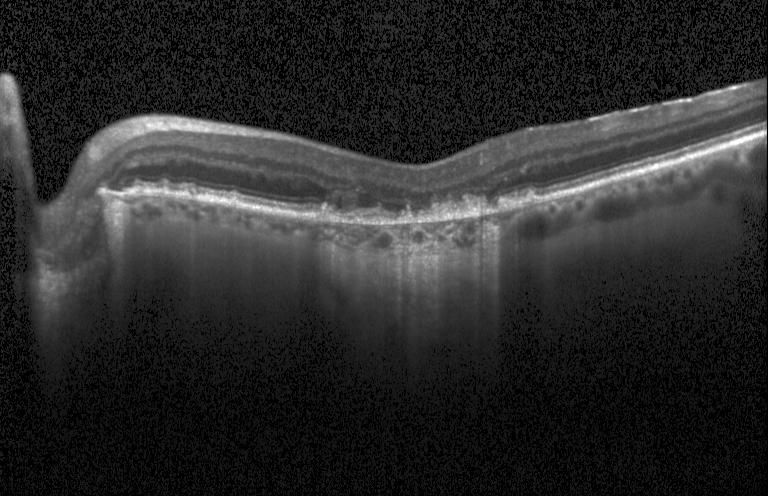
OCT B-scan
Assessment: CNV.